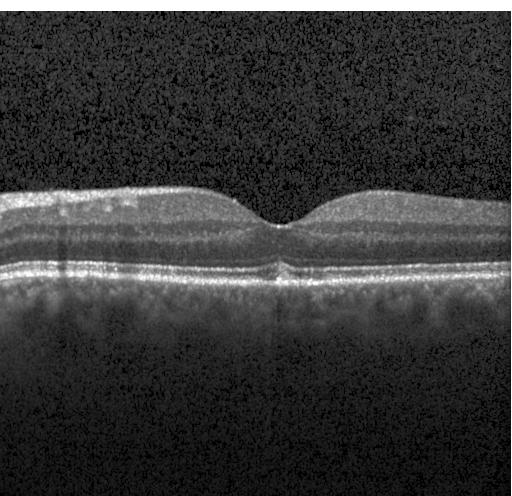 Heidelberg Spectralis OCT system, macular scan, OCT B-scan. Impression: multiple drusen.